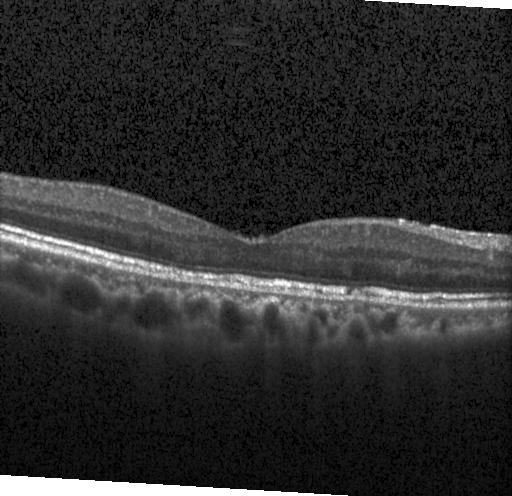

Horizontal scan through the fovea · retinal OCT B-scan — The scan shows no CNV, no DME, and no drusen.